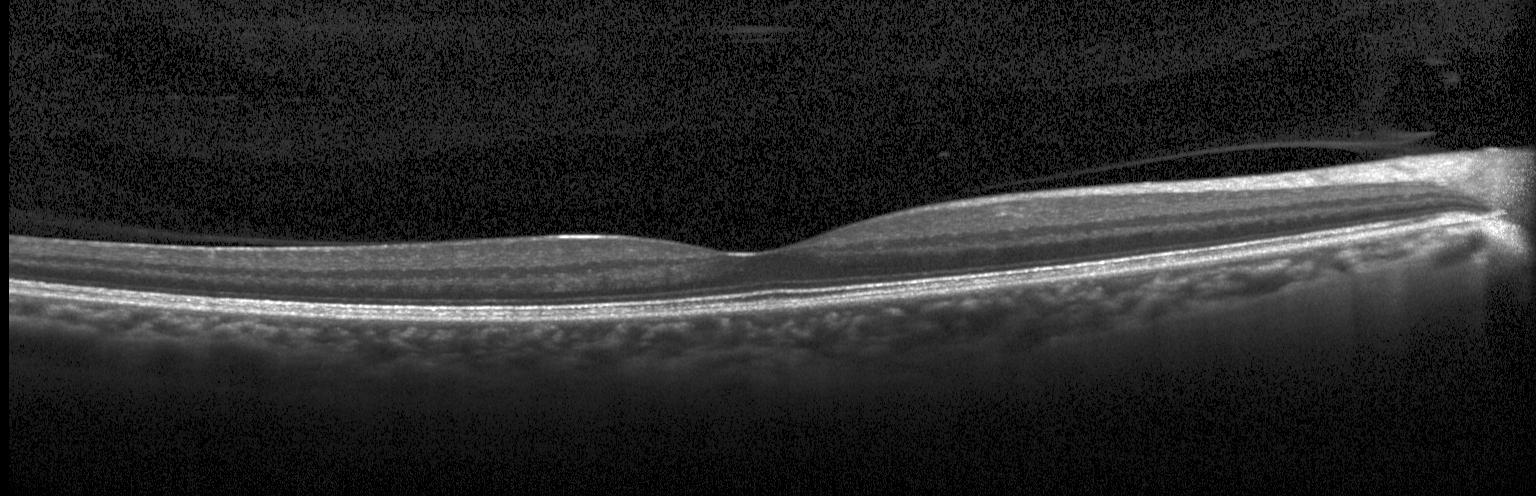
Impression: no CNV, no DME, and no drusen.